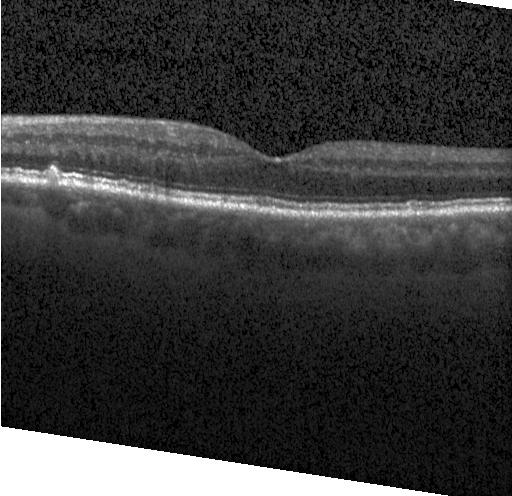
Macular OCT demonstrating sub-RPE drusenoid deposits.